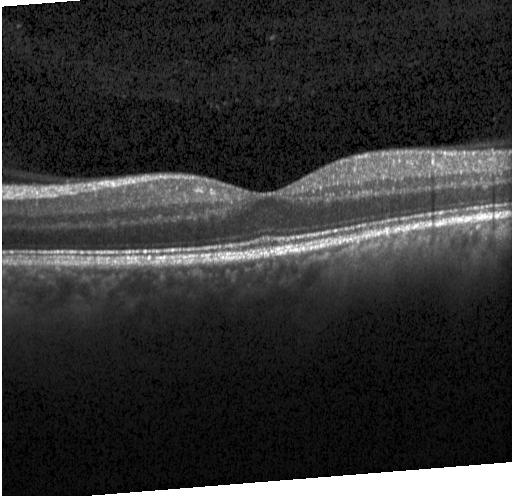
Impression: neither choroidal neovascularization, diabetic macular edema, nor drusen.